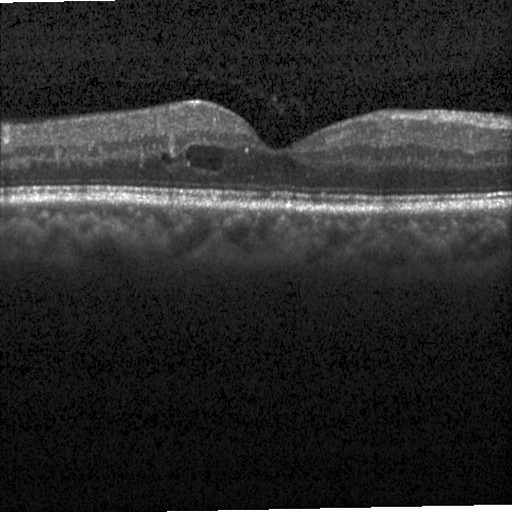

Optical coherence tomography B-scan — OCT finding: diabetic macular edema.